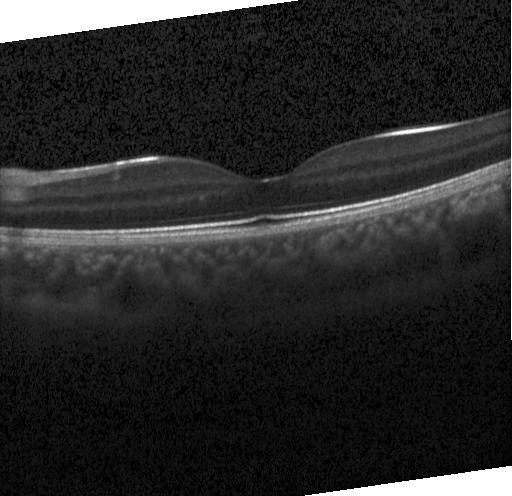

Spectral-domain OCT B-scan: no CNV, no DME, and no drusen.